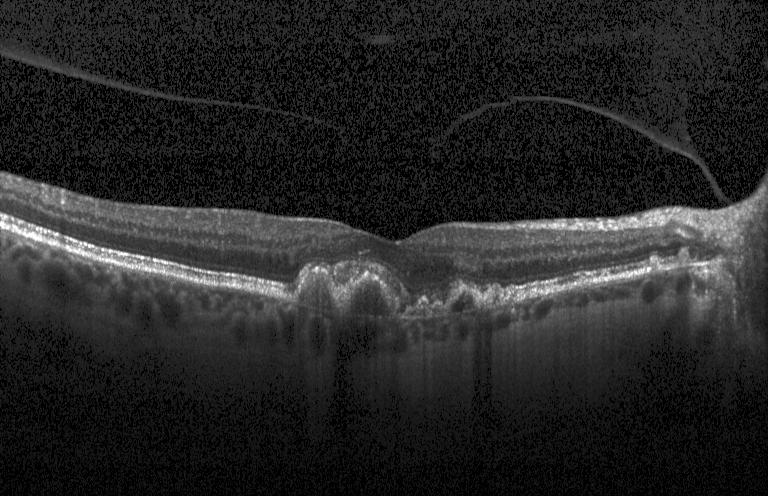 Assessment: CNV.